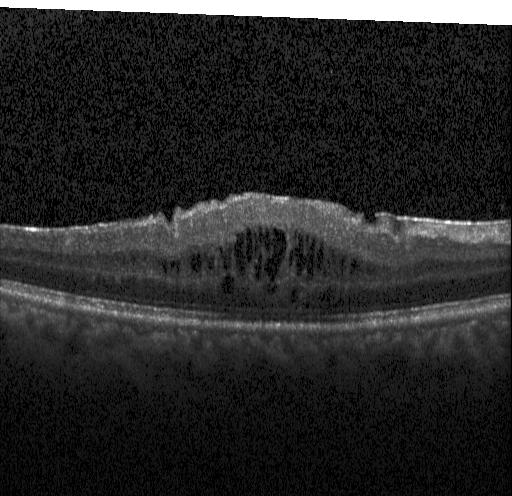

Spectral-domain optical coherence tomography · optical coherence tomography scan
Impression: DME.